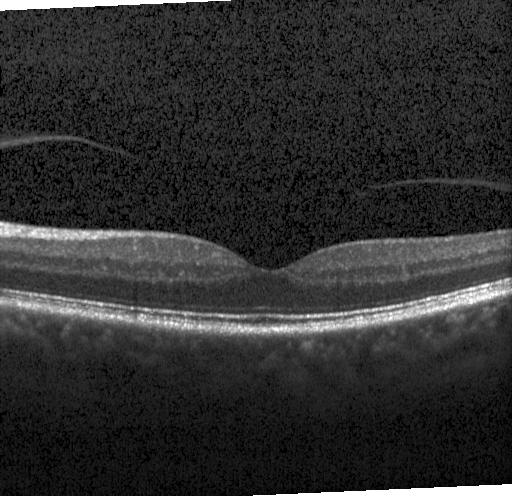 Instrument: Heidelberg Spectralis · fovea-centered · OCT B-scan.
Finding: no choroidal neovascularization, no diabetic macular edema, and no drusen.